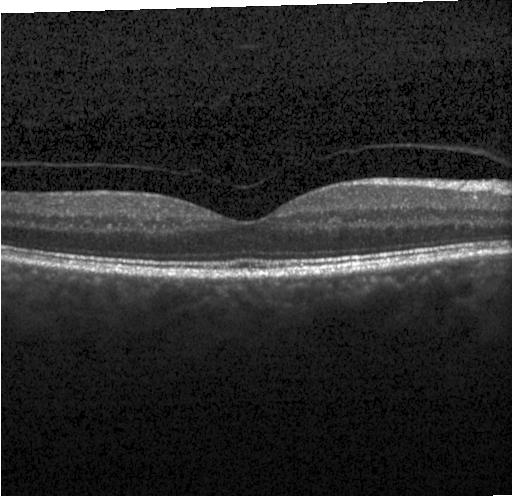
Finding: no choroidal neovascularization, diabetic macular edema, or drusen.